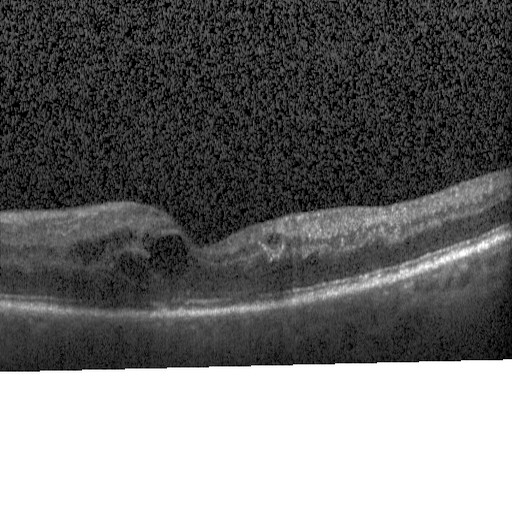

SD-OCT, retinal OCT B-scan, instrument: Heidelberg Spectralis, centered on the fovea.
Diabetic macular edema.